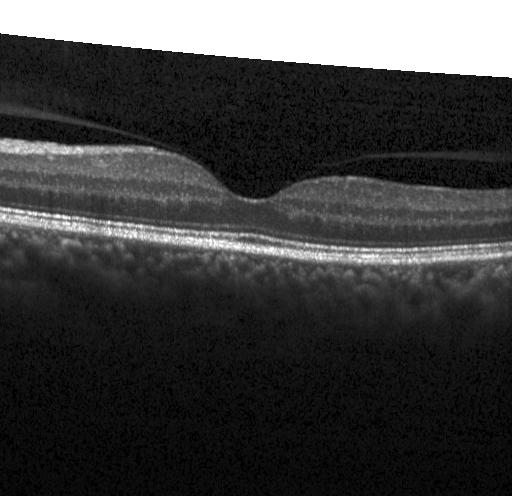

Optical coherence tomography B-scan
Diagnosis: neither choroidal neovascularization, diabetic macular edema, nor drusen.